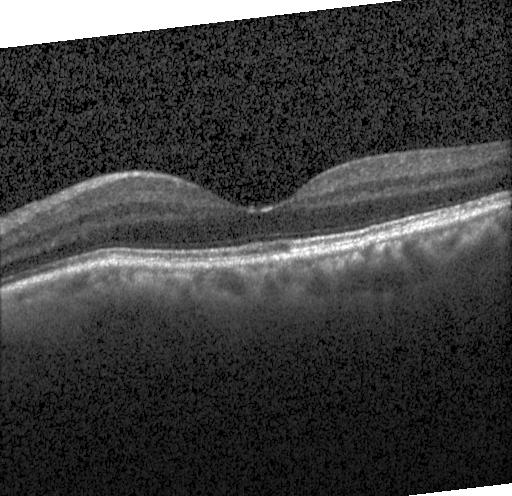 Retinal OCT B-scan.
Assessment: no evidence of choroidal neovascularization, diabetic macular edema, or drusen.